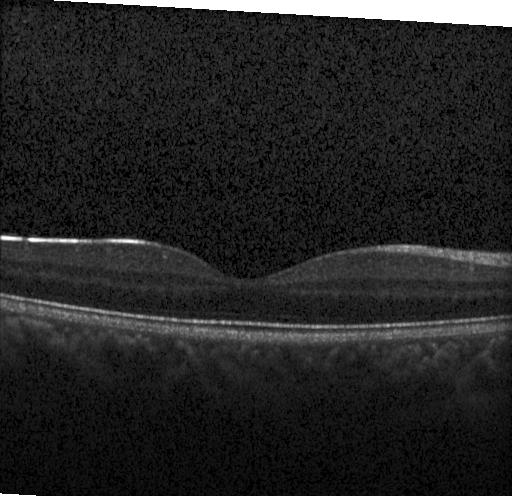
Retinal OCT cross-section showing neither choroidal neovascularization, diabetic macular edema, nor drusen.